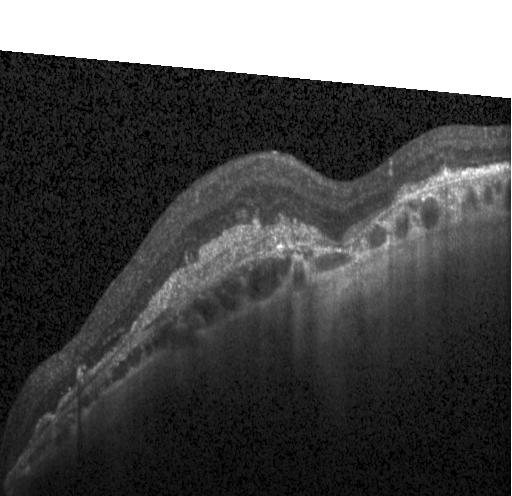 Dx: a choroidal neovascular membrane.